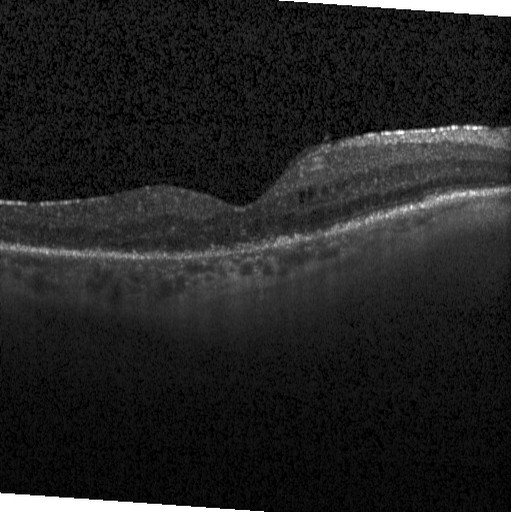

Diagnosis: diabetic macular edema.